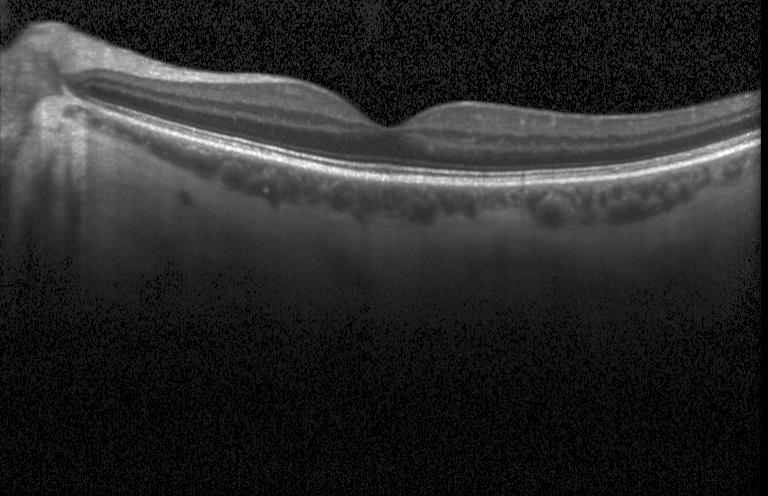 OCT line scan.
The scan shows no choroidal neovascularization, diabetic macular edema, or drusen.